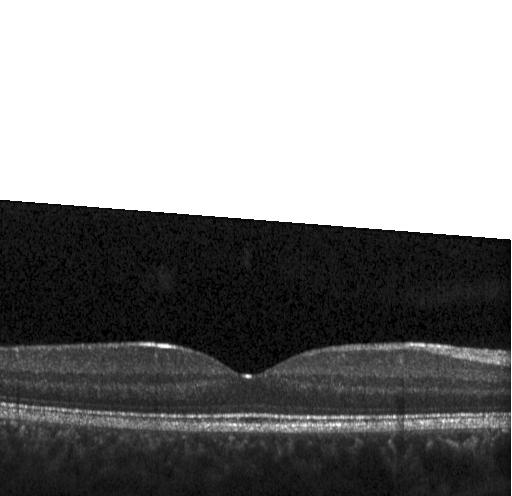 Heidelberg Spectralis · optical coherence tomography scan. Assessment: no evidence of choroidal neovascularization, diabetic macular edema, or drusen.